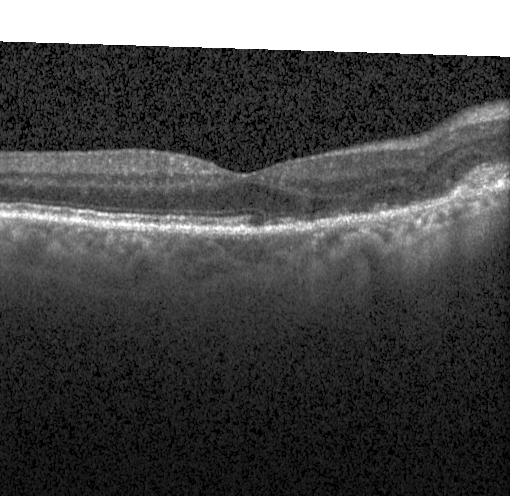 Spectral-domain OCT B-scan: a choroidal neovascular membrane.